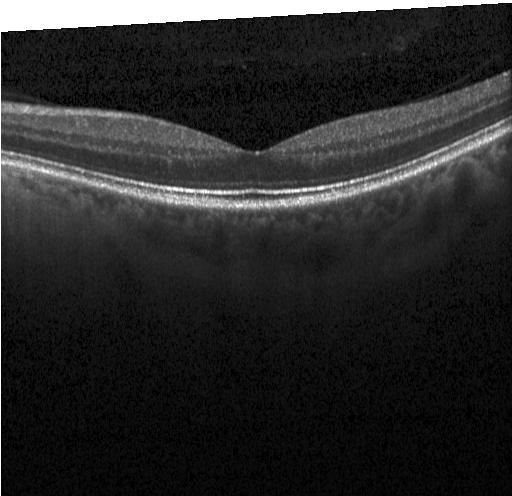 Finding: no evidence of choroidal neovascularization, diabetic macular edema, or drusen.